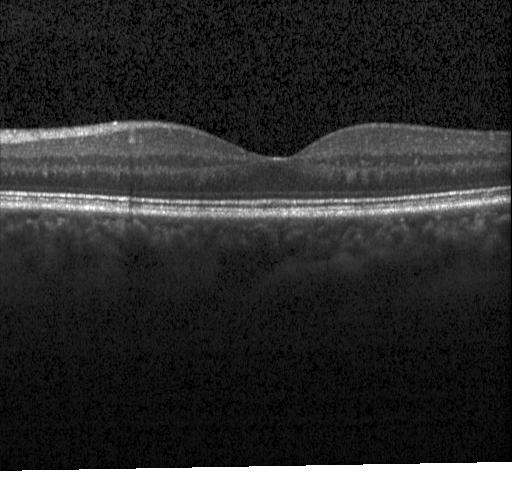
Instrument: Heidelberg Spectralis, through the macula, OCT B-scan. Finding: neither choroidal neovascularization, diabetic macular edema, nor drusen.